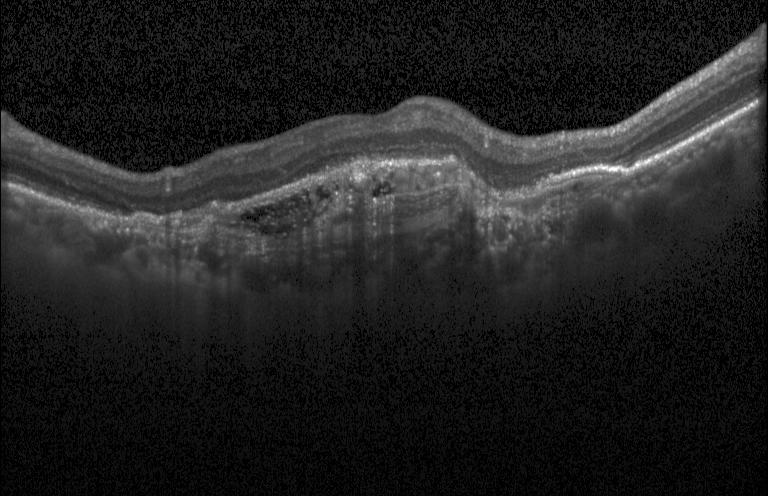

Finding: a choroidal neovascular membrane.